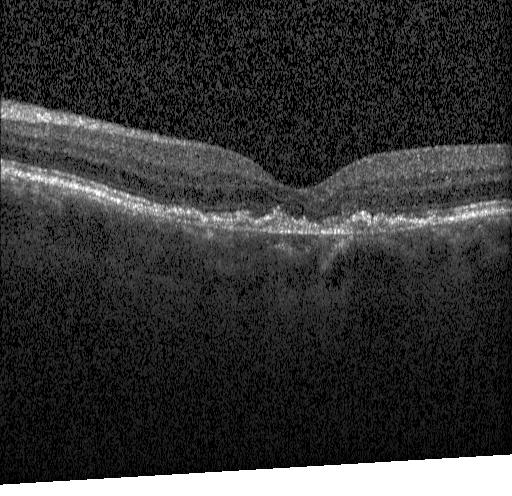 Finding: choroidal neovascularization (CNV).